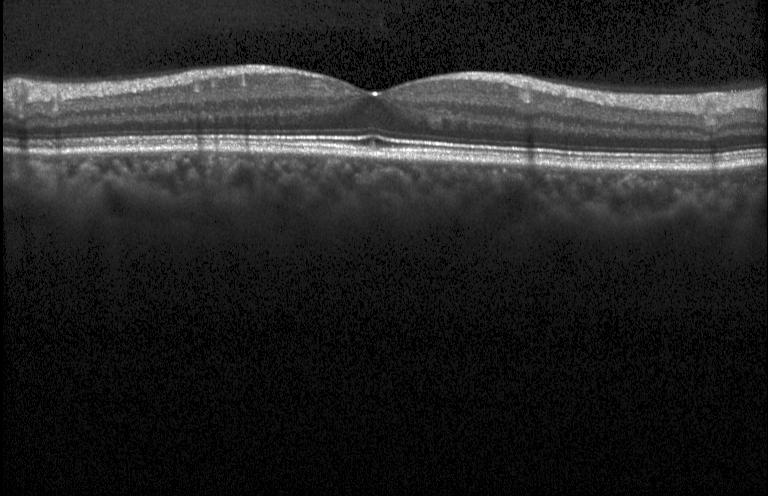
Optical coherence tomography scan, spectral-domain optical coherence tomography.
Macular OCT: no CNV, DME, or drusen.